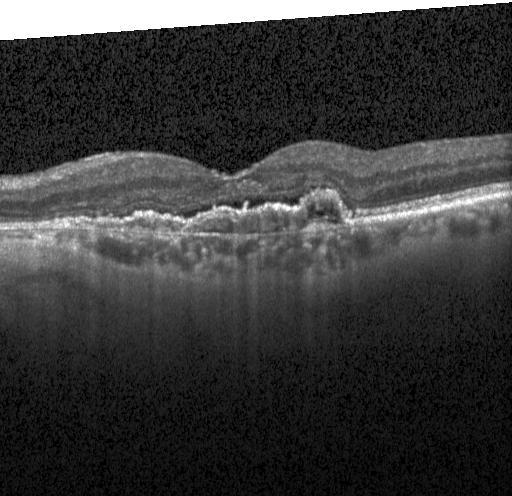
Instrument: Heidelberg Spectralis · SD-OCT · macular scan · OCT line scan
The scan shows CNV.